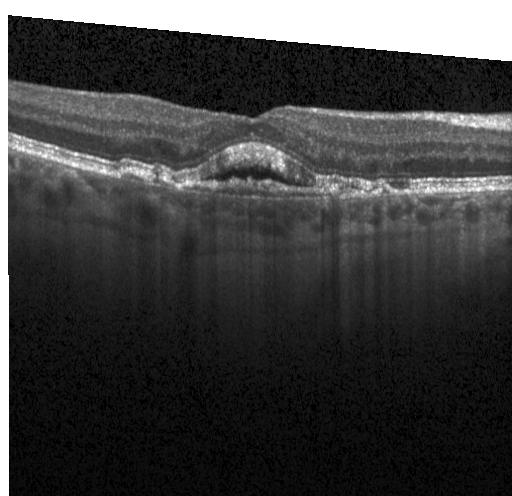 Instrument: Heidelberg Spectralis · optical coherence tomography scan
The scan shows a choroidal neovascular membrane.